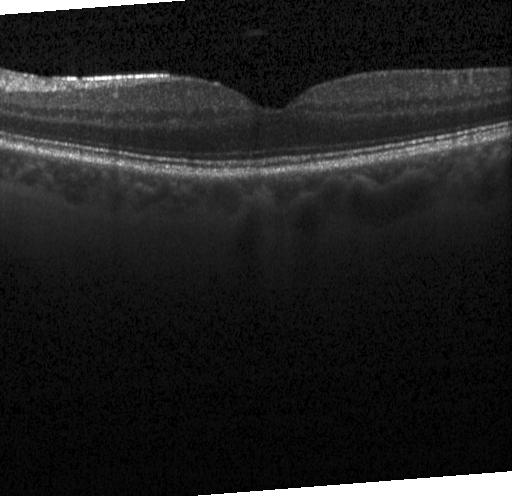

Finding: no CNV, DME, or drusen.